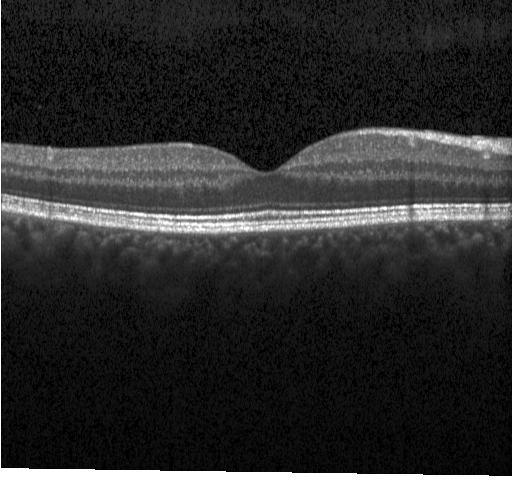

Heidelberg Spectralis OCT system, spectral-domain OCT, optical coherence tomography B-scan
Assessment: no CNV, no DME, and no drusen.